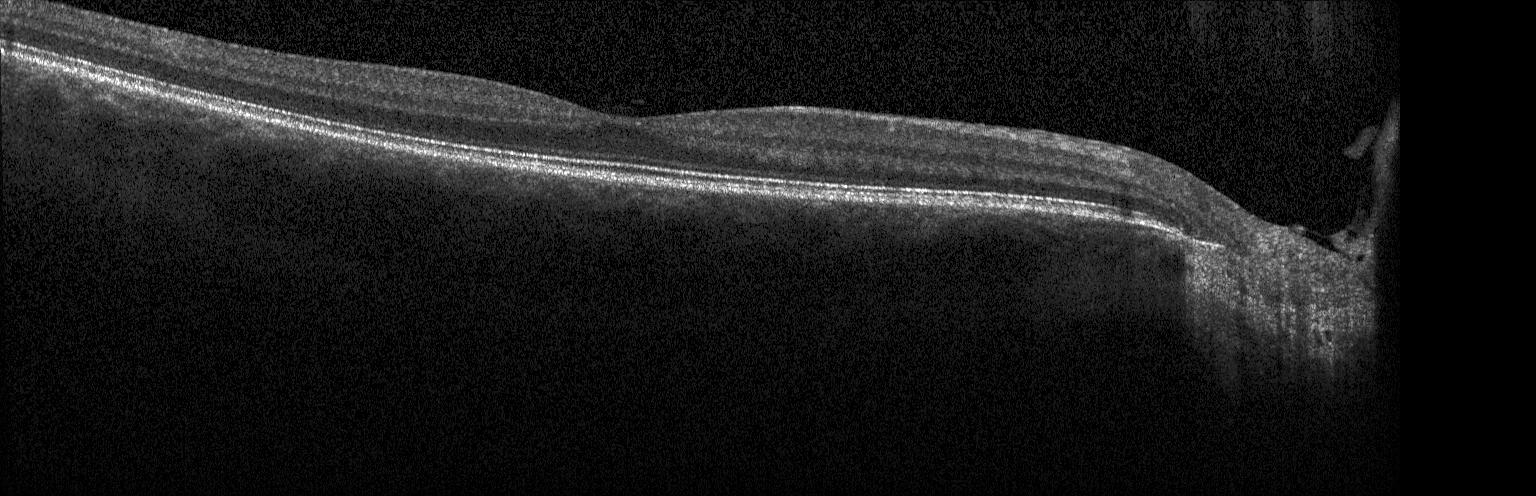 Optical coherence tomography B-scan; spectral-domain optical coherence tomography.
Diagnosis: no choroidal neovascularization, diabetic macular edema, or drusen.